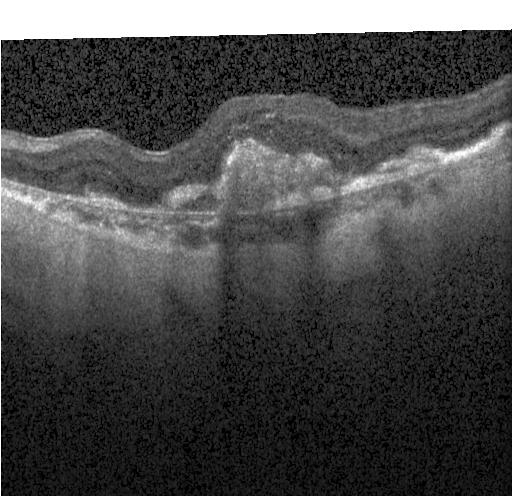

Retinal OCT B-scan — Finding: choroidal neovascularization.